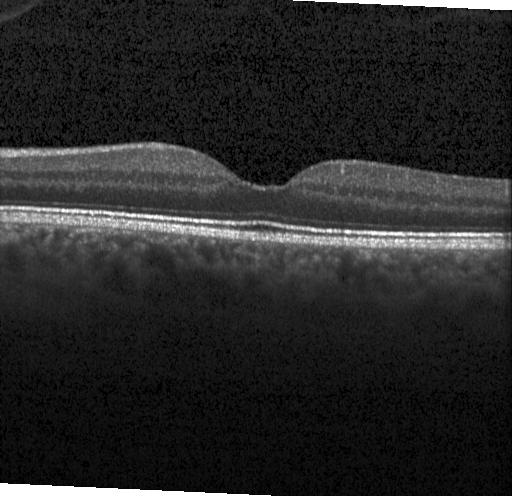
OCT B-scan; horizontal scan through the fovea; instrument: Heidelberg Spectralis.
Impression: neither choroidal neovascularization, diabetic macular edema, nor drusen.